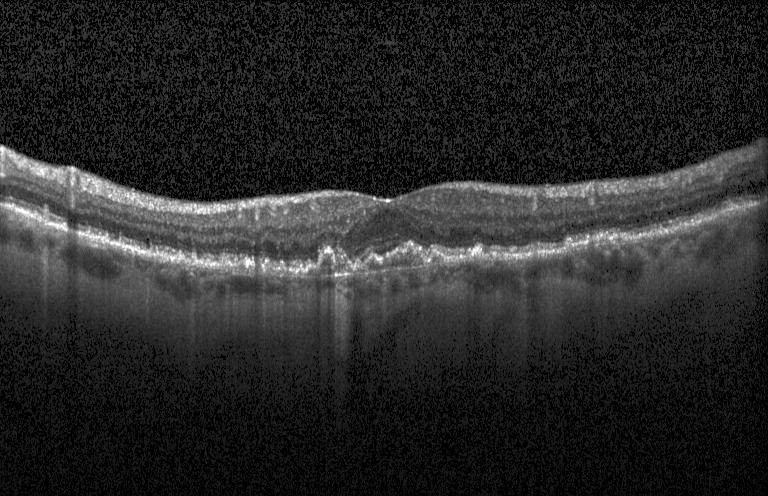

Retinal OCT B-scan. Instrument: Heidelberg Spectralis. Horizontal scan through the fovea
Diagnosis: a choroidal neovascular membrane.